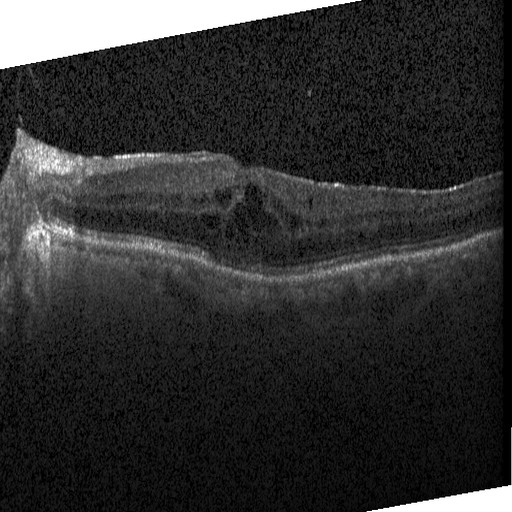
Optical coherence tomography B-scan. Centered on the fovea. Acquired on a Heidelberg Spectralis. Macular OCT: DME.